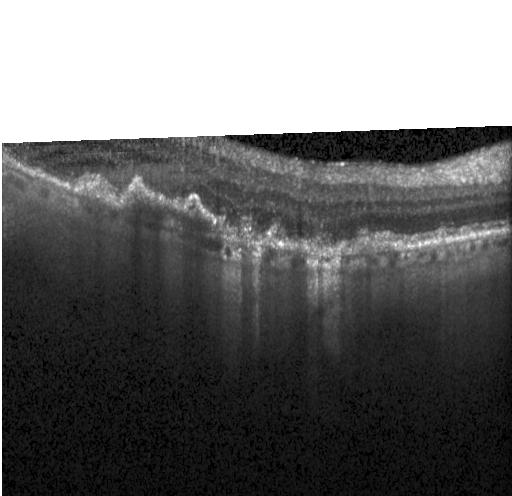

Optical coherence tomography scan. Instrument: Heidelberg Spectralis. Macular scan
Finding: choroidal neovascularization (CNV).